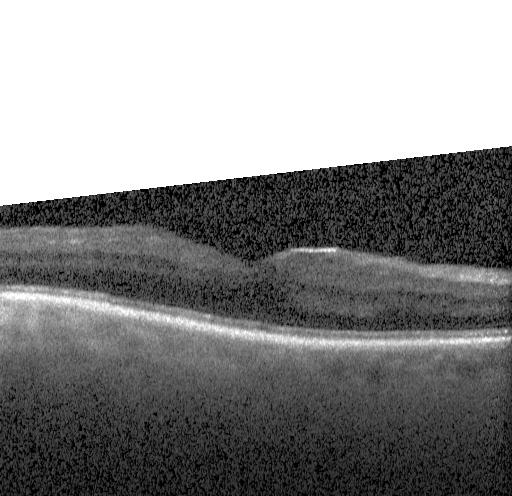 OCT line scan. Macular OCT: no choroidal neovascularization, no diabetic macular edema, and no drusen.